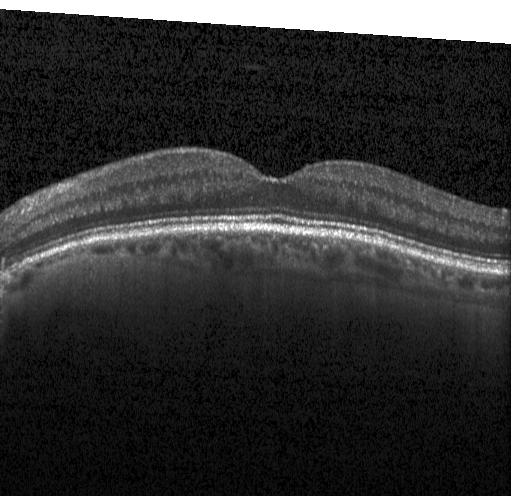 OCT B-scan — Finding: no evidence of CNV, DME, or drusen.